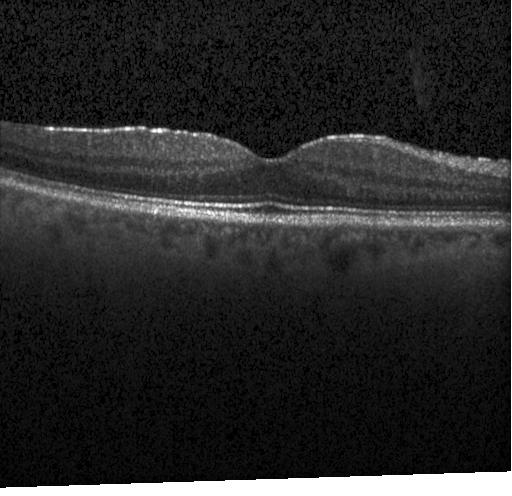
Fovea-centered. Retinal OCT B-scan. Heidelberg Spectralis OCT system.
The scan shows no choroidal neovascularization, no diabetic macular edema, and no drusen.